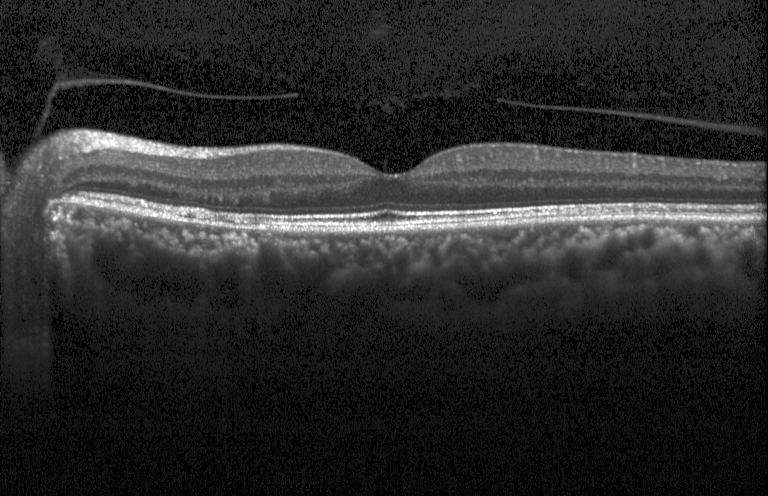

Impression: no choroidal neovascularization, diabetic macular edema, or drusen.